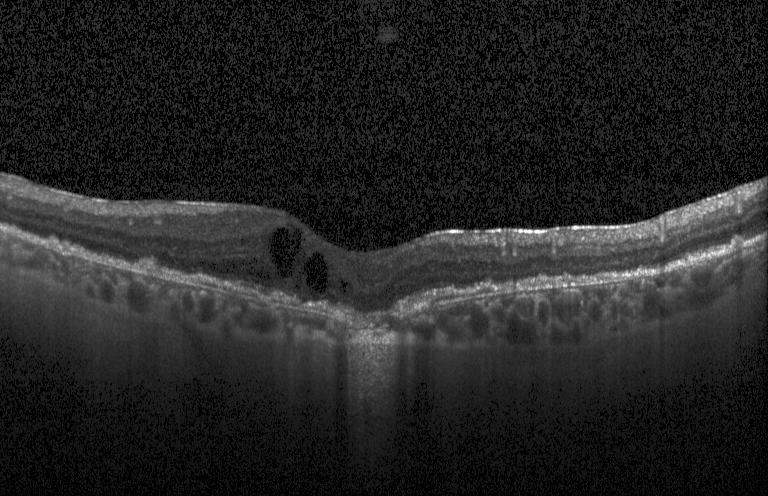

OCT line scan
Diagnosis: a choroidal neovascular membrane.